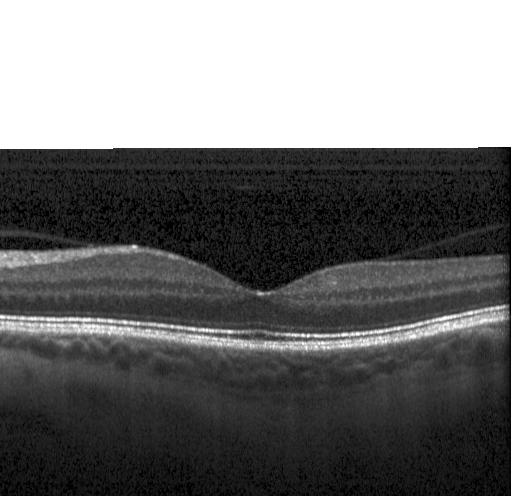 Macular OCT demonstrating neither choroidal neovascularization, diabetic macular edema, nor drusen.